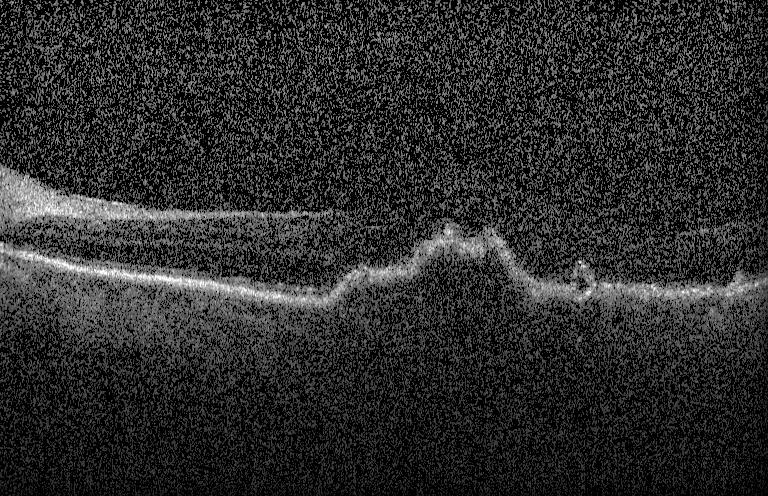 Instrument: Heidelberg Spectralis, retinal OCT cross-section, centered on the fovea, spectral-domain optical coherence tomography.
Impression: a choroidal neovascular membrane.